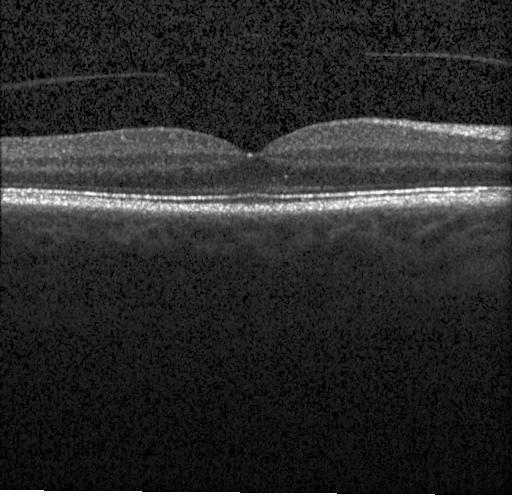
Optical coherence tomography scan.
OCT finding: no CNV, no DME, and no drusen.